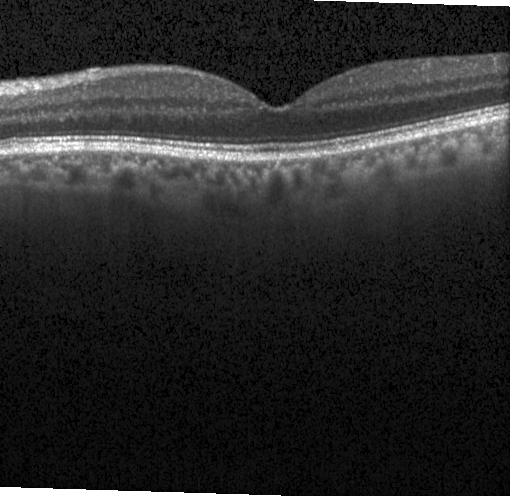
This B-scan demonstrates no evidence of choroidal neovascularization, diabetic macular edema, or drusen.